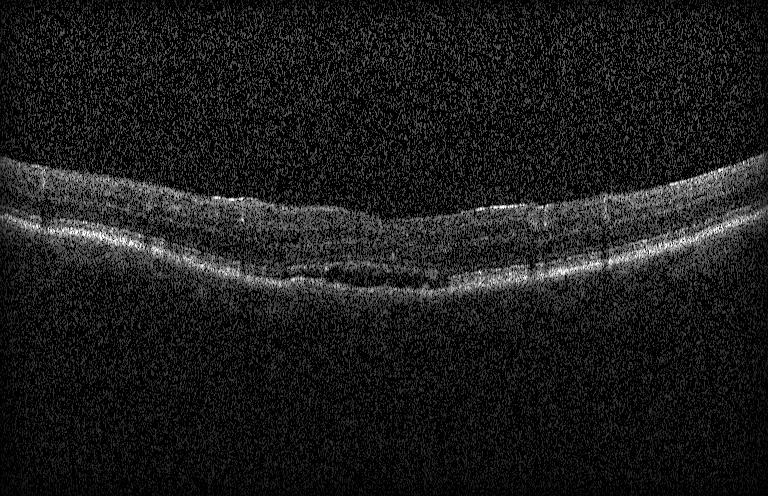

Spectral-domain OCT, retinal OCT B-scan, Heidelberg Spectralis, fovea-centered
Finding: choroidal neovascularization.